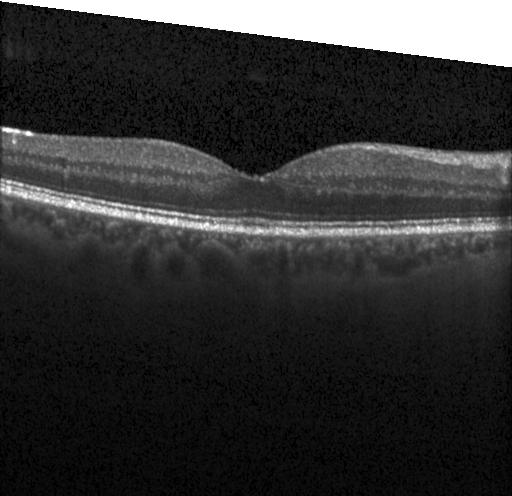
Optical coherence tomography B-scan — Impression: neither CNV, DME, nor drusen.